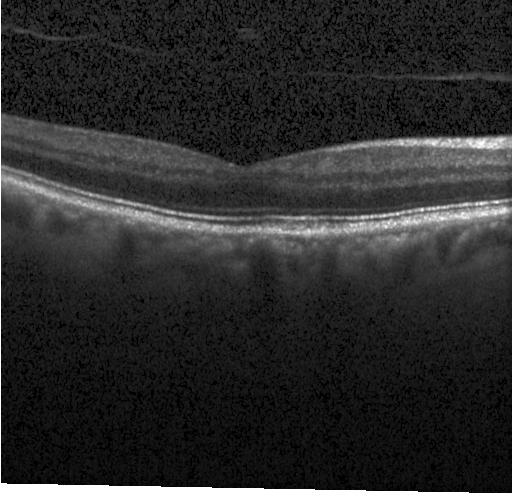

Horizontal scan through the fovea · Heidelberg Spectralis · optical coherence tomography scan. This B-scan demonstrates no CNV, no DME, and no drusen.